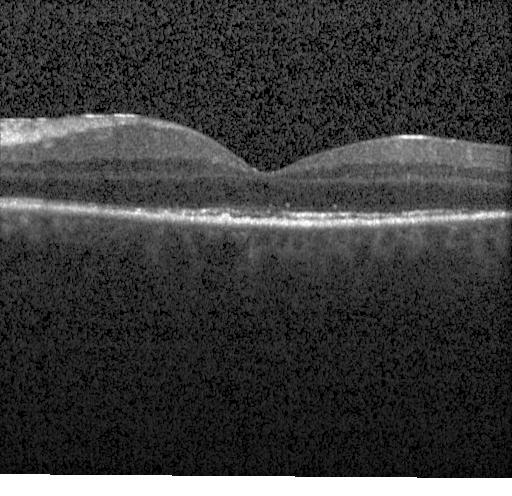

Through the macula, retinal OCT cross-section, instrument: Heidelberg Spectralis, spectral-domain optical coherence tomography.
No evidence of CNV, DME, or drusen.